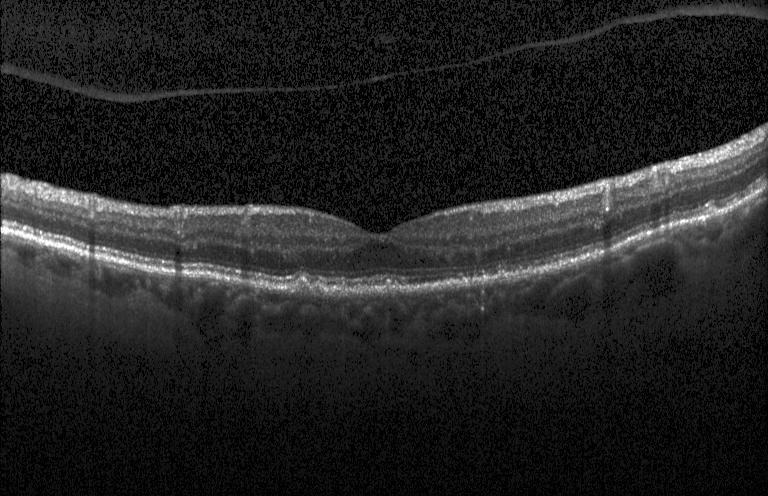

SD-OCT; Heidelberg Spectralis OCT system; optical coherence tomography B-scan; through the macula.
Drusen.